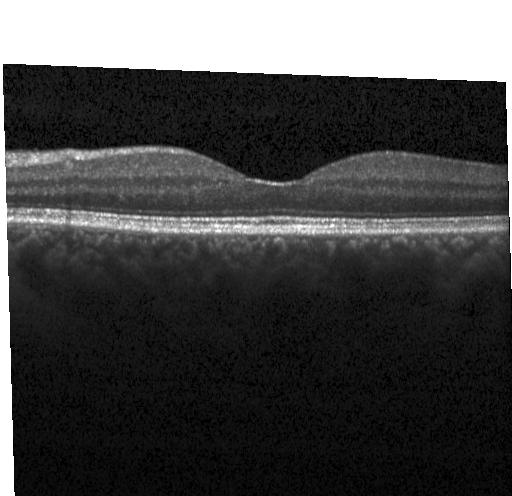 OCT scan showing no choroidal neovascularization, no diabetic macular edema, and no drusen.